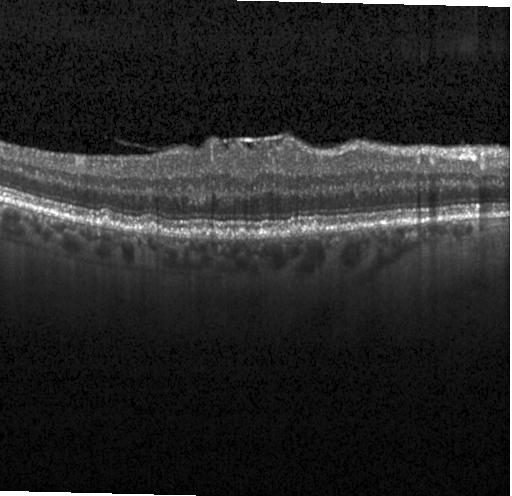

Impression: multiple drusen.